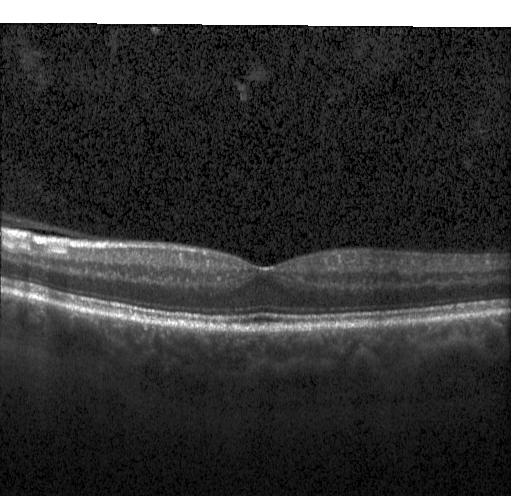
Spectral-domain OCT. Macular scan. OCT B-scan. Instrument: Heidelberg Spectralis
This B-scan demonstrates no evidence of choroidal neovascularization, diabetic macular edema, or drusen.